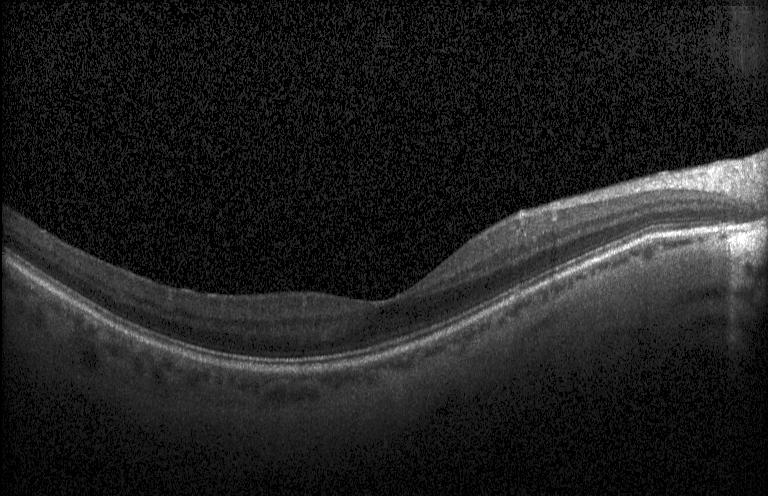

Optical coherence tomography B-scan
Dx: no evidence of choroidal neovascularization, diabetic macular edema, or drusen.